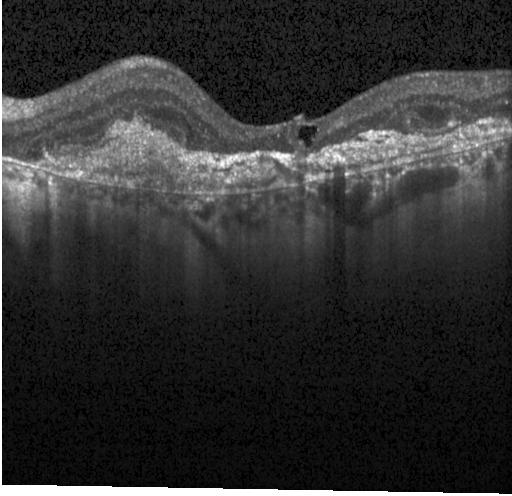

OCT B-scan · SD-OCT · centered on the fovea · Heidelberg Spectralis OCT system — Diagnosis: a choroidal neovascular membrane.